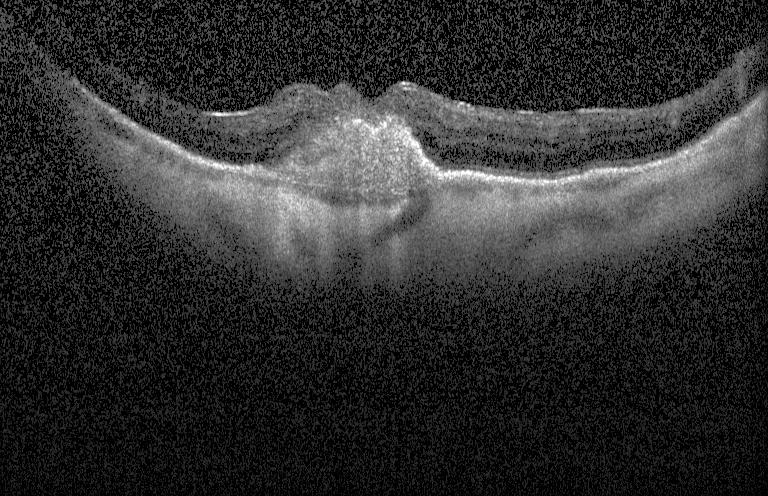

Instrument: Heidelberg Spectralis. Spectral-domain OCT. Through the macula. OCT line scan.
The scan shows a choroidal neovascular membrane.